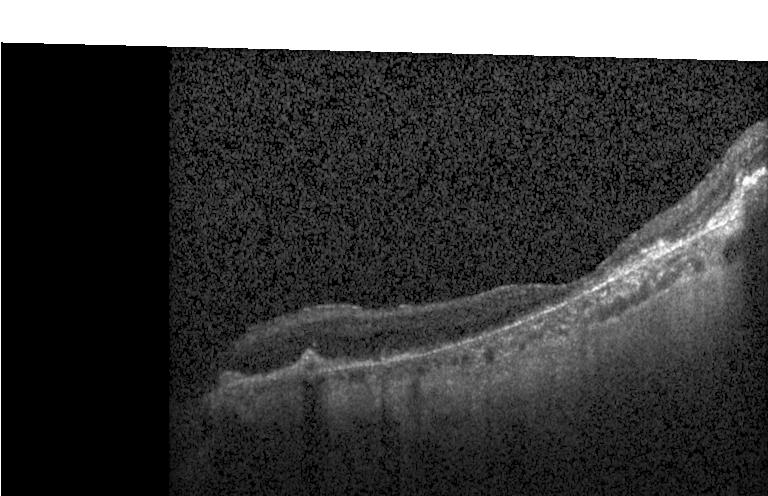
Finding: CNV.